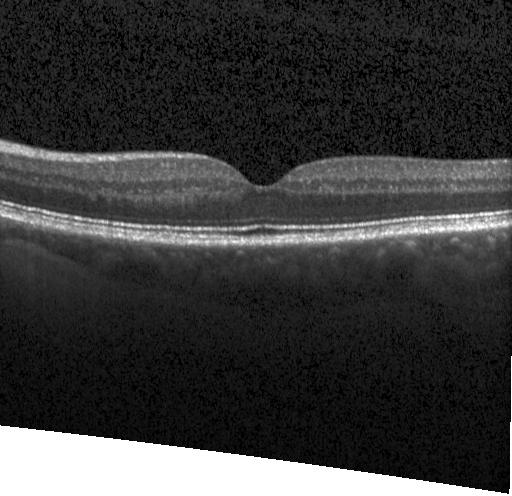 No evidence of choroidal neovascularization, diabetic macular edema, or drusen.